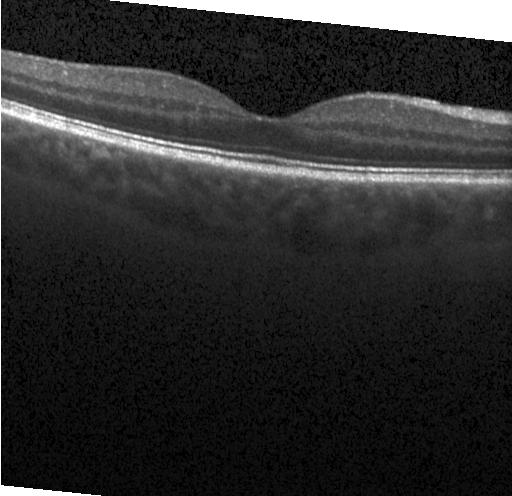

Retinal OCT cross-section.
Diagnosis: no choroidal neovascularization, diabetic macular edema, or drusen.